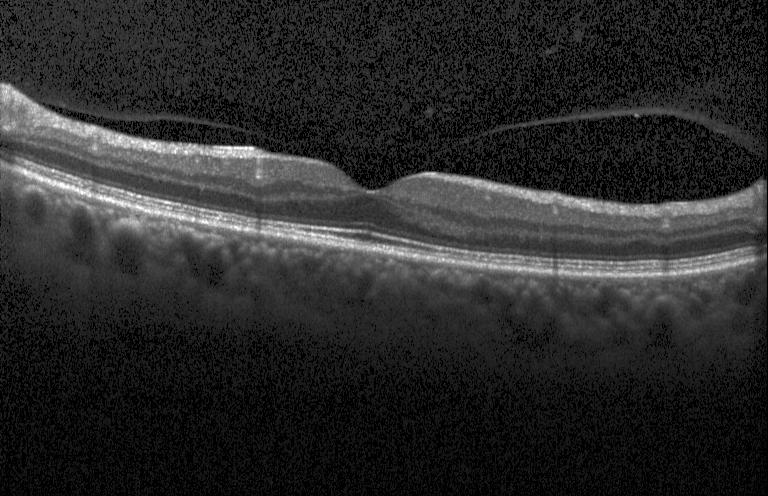

Assessment: no CNV, DME, or drusen.